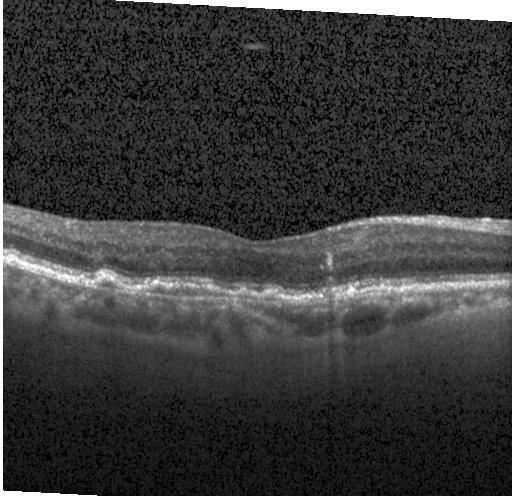

Macular OCT: a choroidal neovascular membrane.